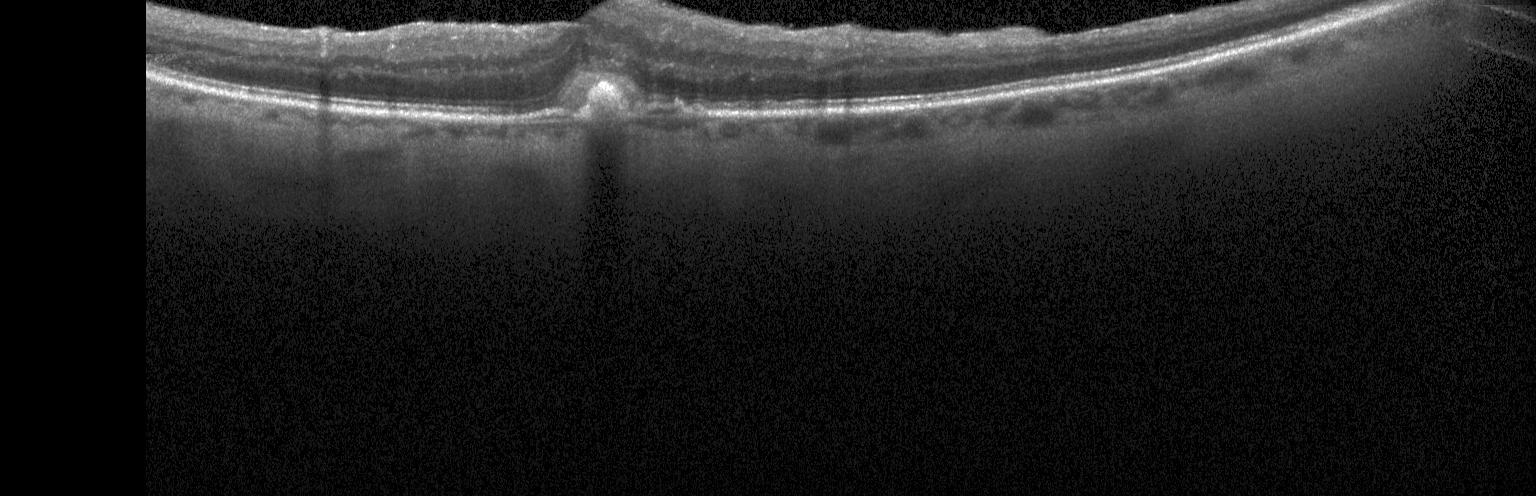
Macular OCT demonstrating CNV.